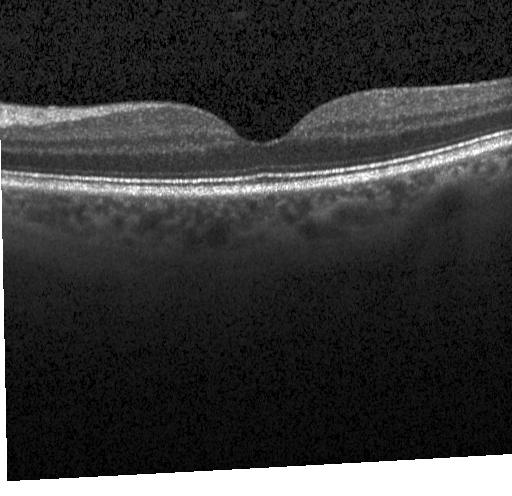

Heidelberg Spectralis OCT system. SD-OCT. OCT B-scan. Through the macula — Diagnosis: no choroidal neovascularization, diabetic macular edema, or drusen.